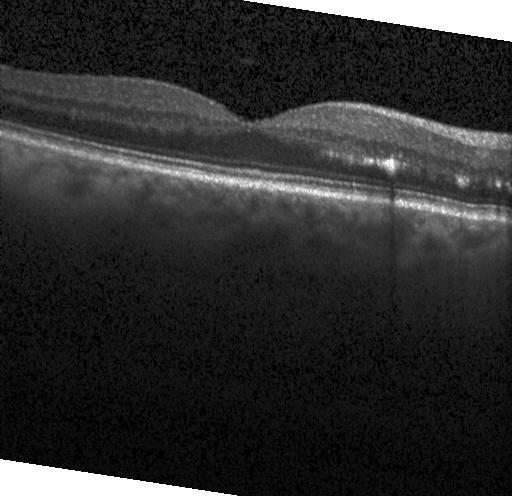

Optical coherence tomography scan; acquired on a Heidelberg Spectralis — Diagnosis: no evidence of choroidal neovascularization, diabetic macular edema, or drusen.